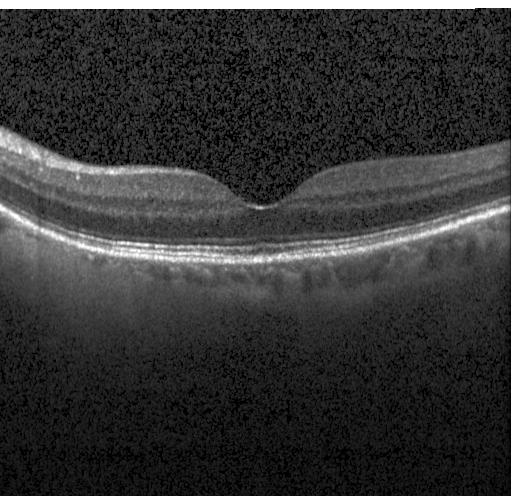 Heidelberg Spectralis OCT system. SD-OCT. Retinal OCT B-scan. Fovea-centered — Finding: no CNV, no DME, and no drusen.